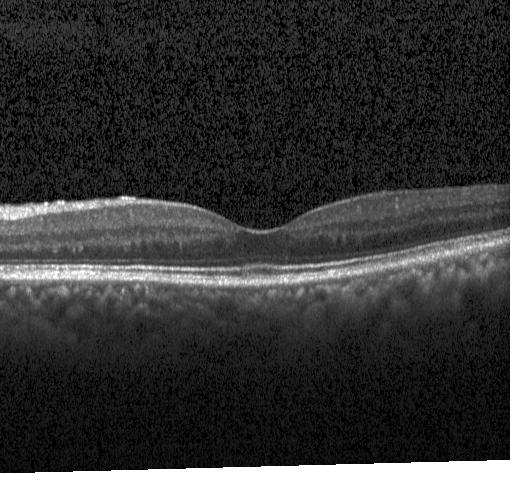

Retinal OCT cross-section.
Diagnosis: no evidence of CNV, DME, or drusen.